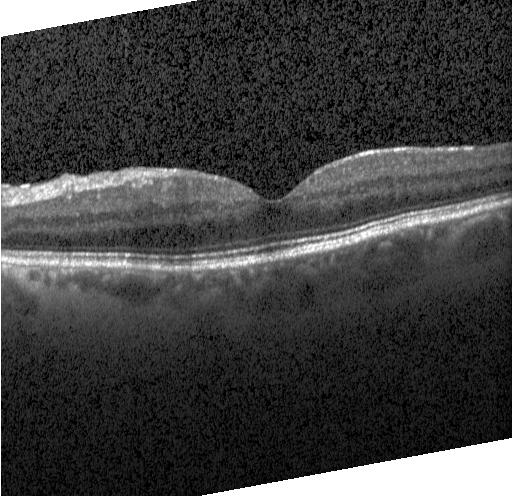 Spectral-domain optical coherence tomography, acquired on a Heidelberg Spectralis, retinal OCT cross-section — Assessment: no choroidal neovascularization, no diabetic macular edema, and no drusen.